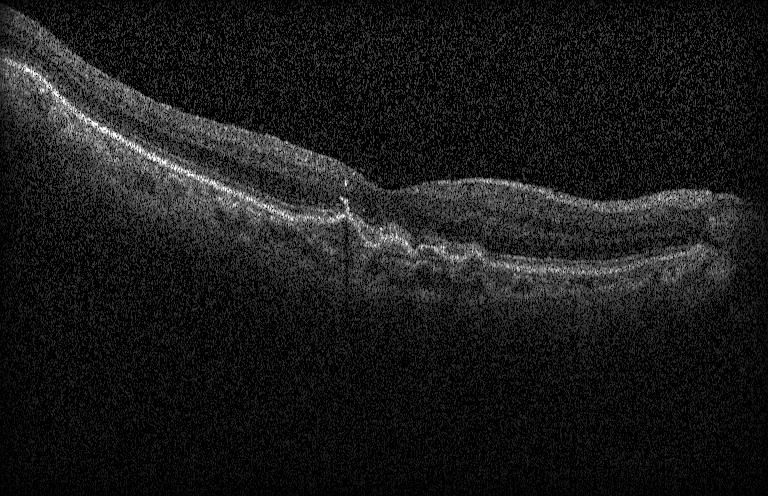
OCT B-scan. Centered on the fovea. Heidelberg Spectralis OCT system. Spectral-domain optical coherence tomography — Finding: choroidal neovascularization.